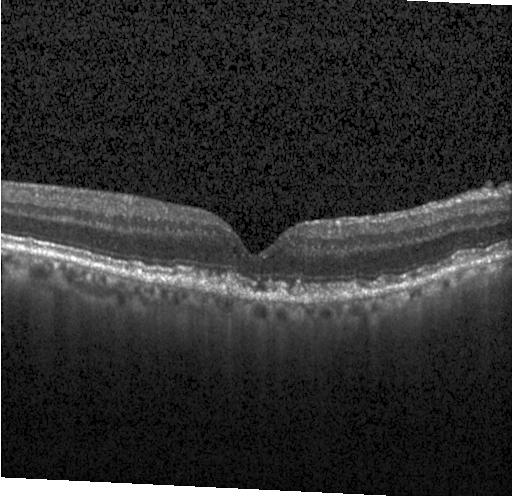 Instrument: Heidelberg Spectralis, retinal OCT cross-section, through the macula. Finding: sub-RPE drusenoid deposits.